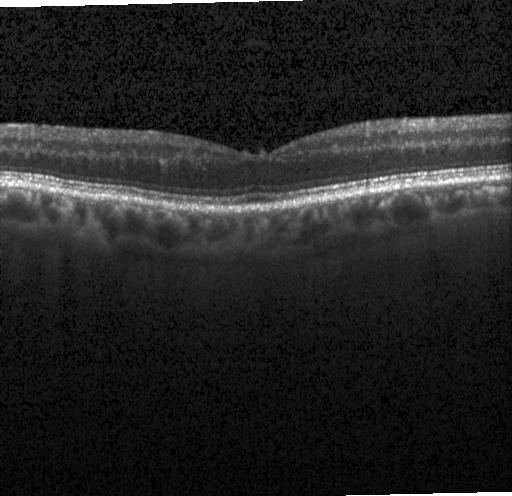
Optical coherence tomography scan, macular scan, Heidelberg Spectralis OCT system, SD-OCT
Diagnosis: neither choroidal neovascularization, diabetic macular edema, nor drusen.